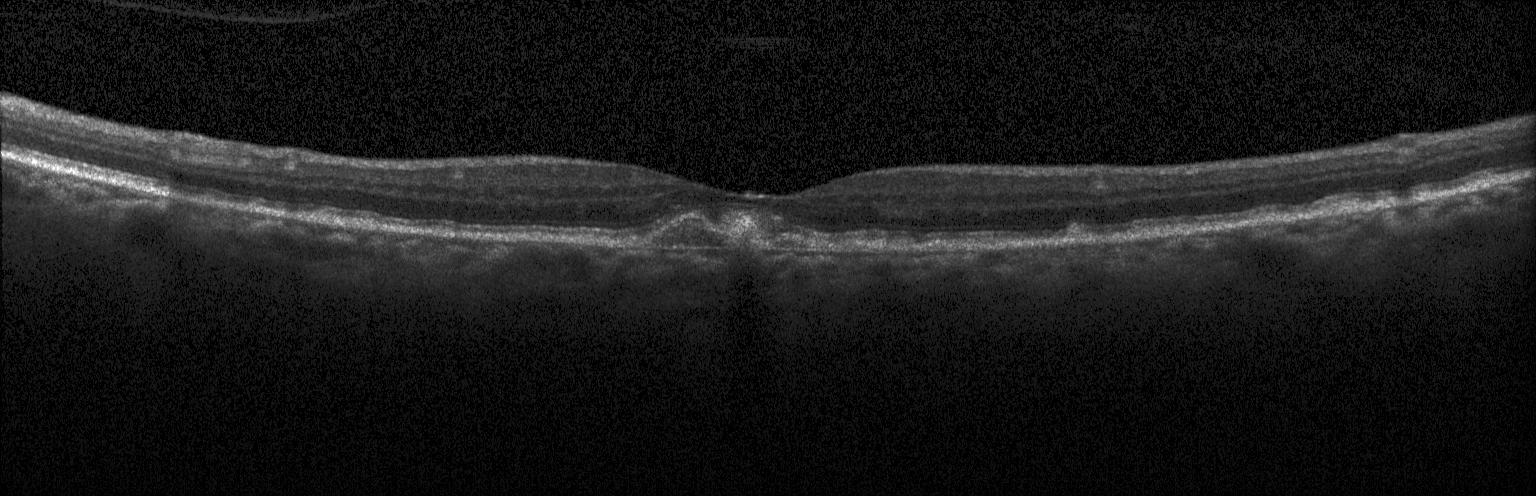

Optical coherence tomography B-scan
Diagnosis: choroidal neovascularization.